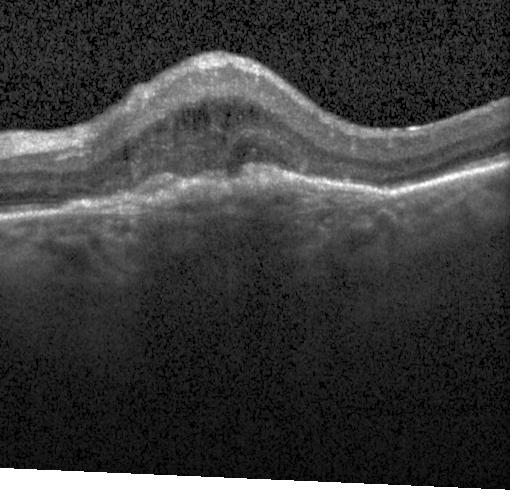
Through the macula. Retinal OCT B-scan
Impression: choroidal neovascularization (CNV).